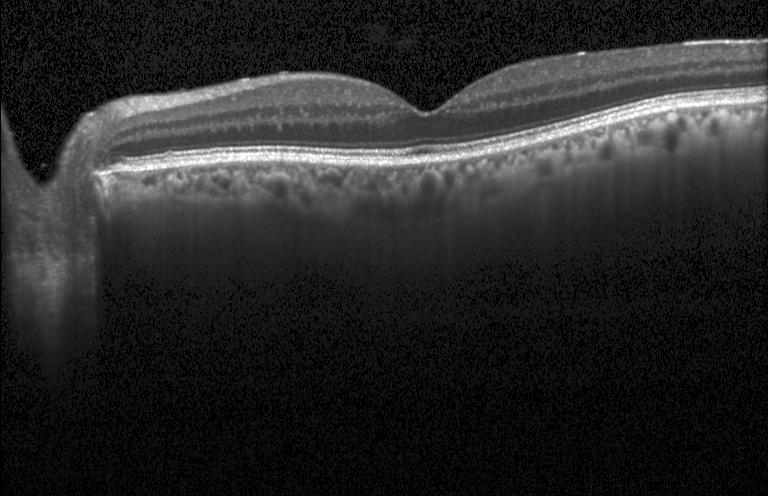 Retinal OCT cross-section. This B-scan demonstrates no choroidal neovascularization, diabetic macular edema, or drusen.